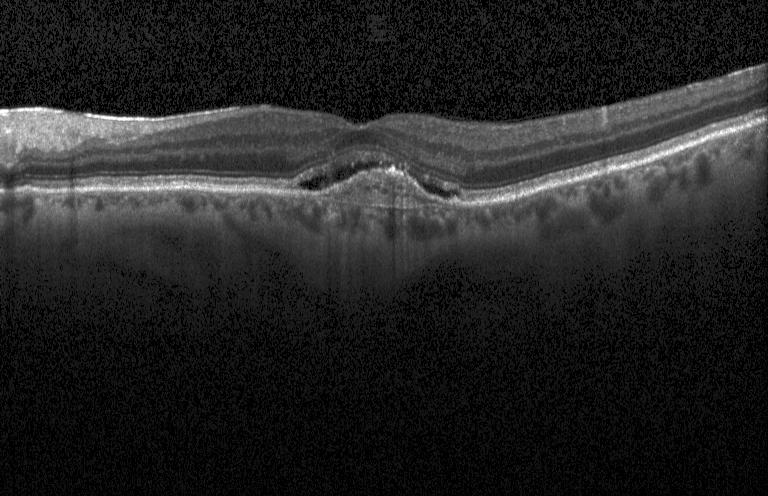 Optical coherence tomography scan. Impression: choroidal neovascularization.